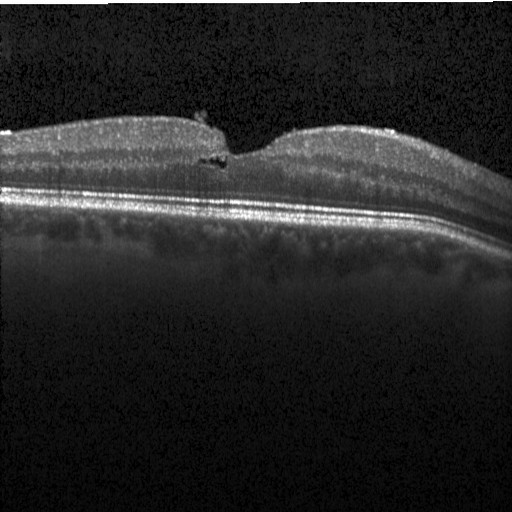
Optical coherence tomography scan
Dx: diabetic macular edema.